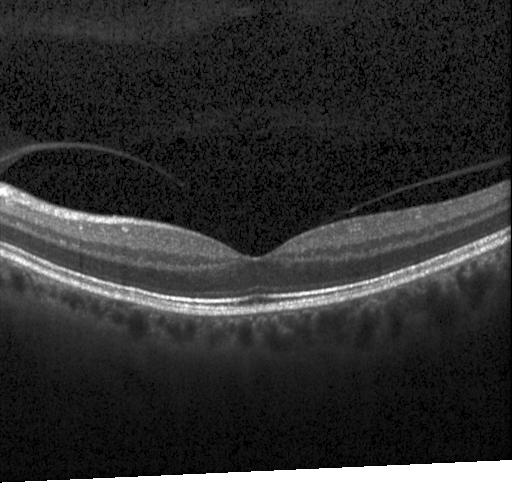
Centered on the fovea, Heidelberg Spectralis, retinal OCT B-scan. Assessment: no choroidal neovascularization, diabetic macular edema, or drusen.